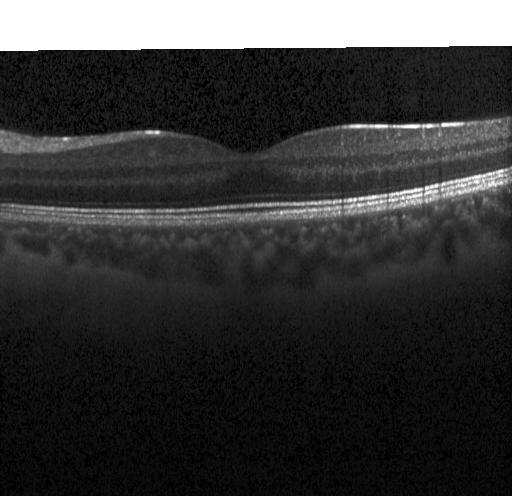
Optical coherence tomography B-scan, centered on the fovea, Heidelberg Spectralis. Macular OCT: no evidence of choroidal neovascularization, diabetic macular edema, or drusen.